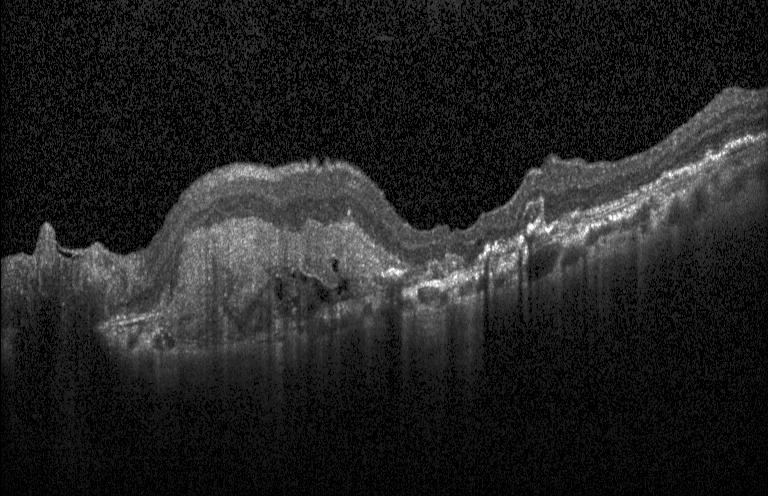

Finding: a choroidal neovascular membrane.